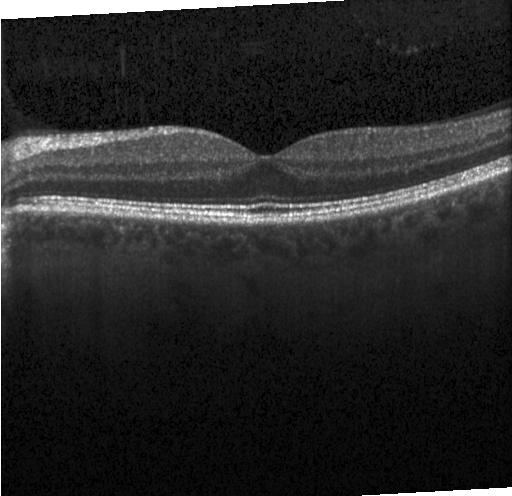

Diagnosis: no evidence of choroidal neovascularization, diabetic macular edema, or drusen.